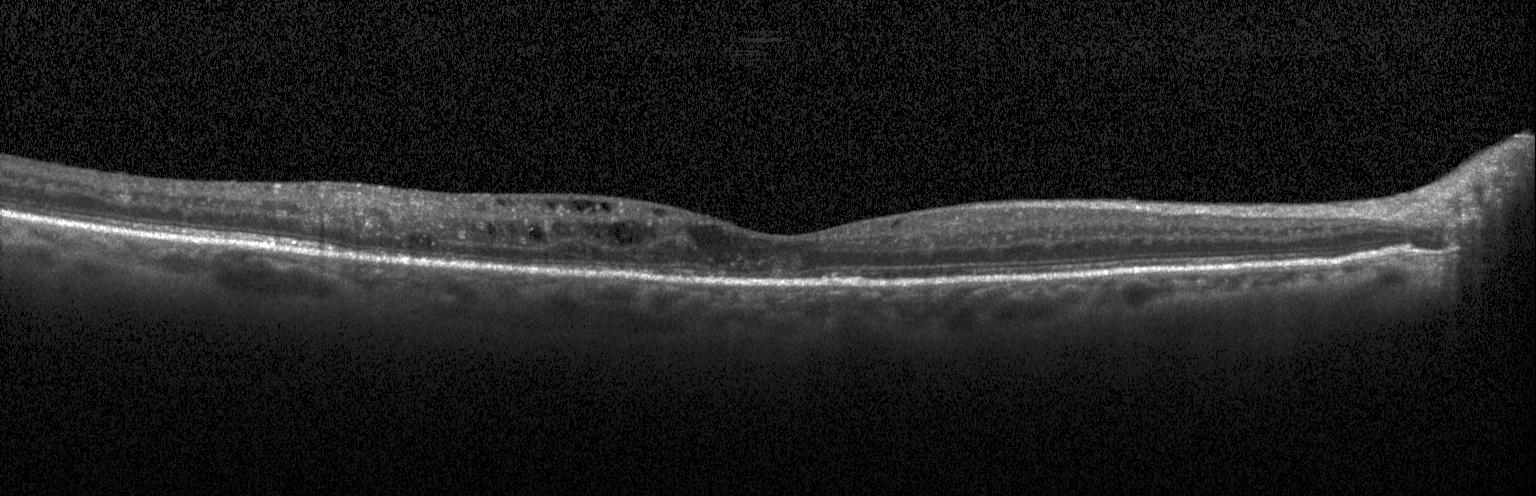 Retinal OCT cross-section showing diabetic macular edema (DME).